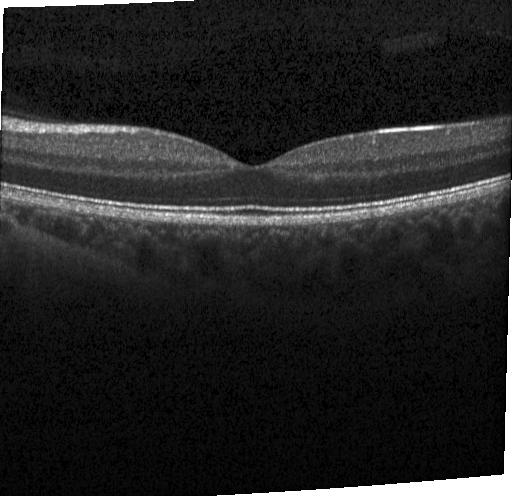

OCT B-scan. Finding: no CNV, no DME, and no drusen.